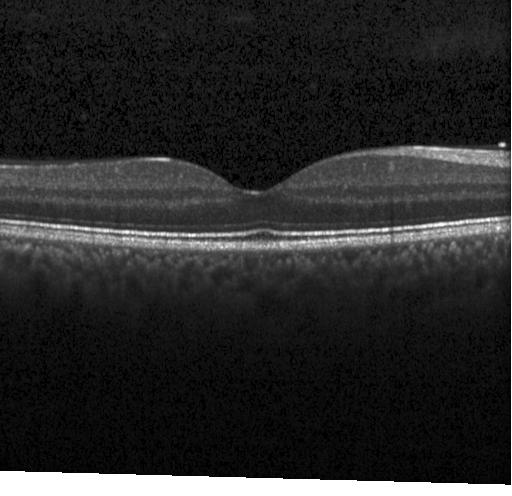 Neither CNV, DME, nor drusen.